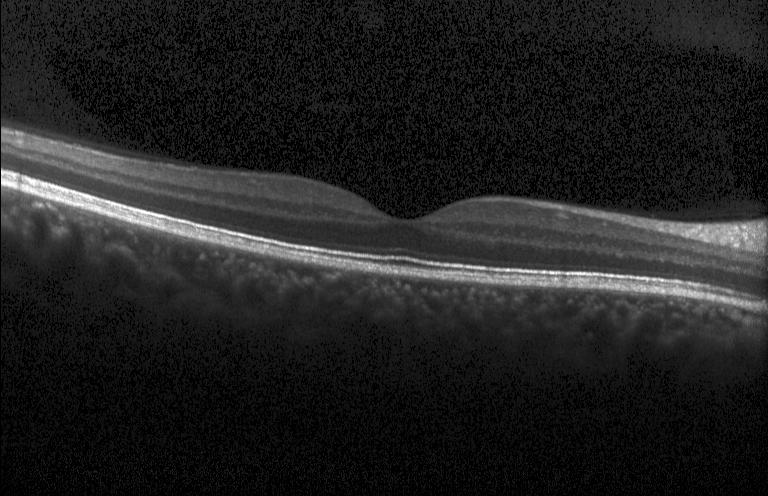 Acquired on a Heidelberg Spectralis · macular scan · OCT line scan. No CNV, no DME, and no drusen.